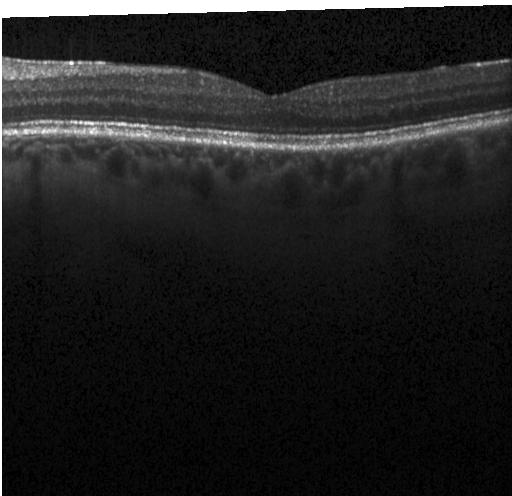

Heidelberg Spectralis; optical coherence tomography B-scan; spectral-domain optical coherence tomography — This B-scan demonstrates no evidence of CNV, DME, or drusen.